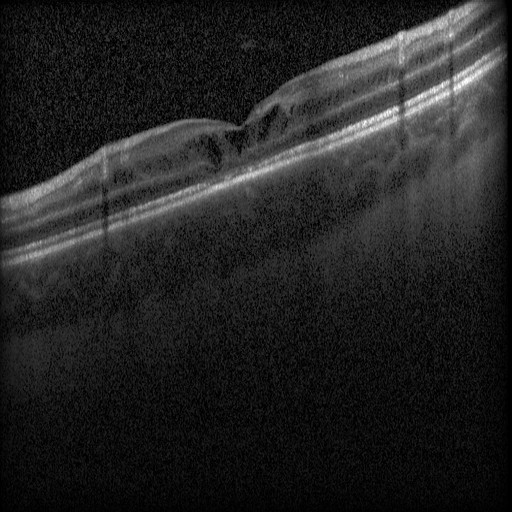 Macular scan. Spectral-domain optical coherence tomography. Optical coherence tomography scan
Finding: DME.